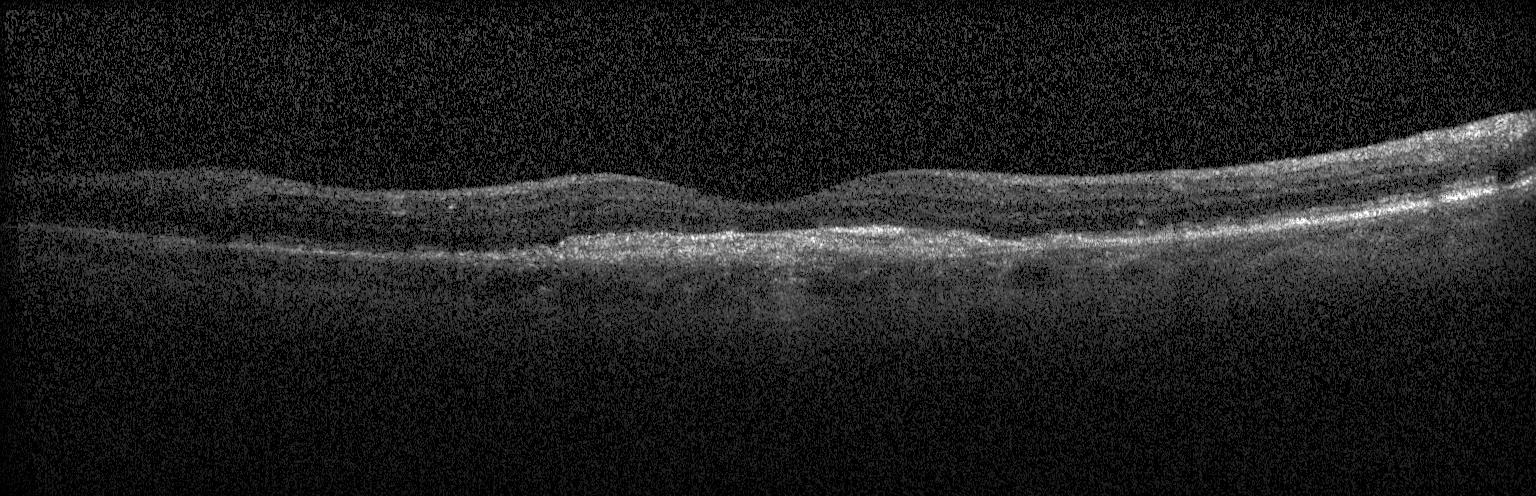
Fovea-centered. Spectral-domain optical coherence tomography. Retinal OCT B-scan
Impression: choroidal neovascularization (CNV).